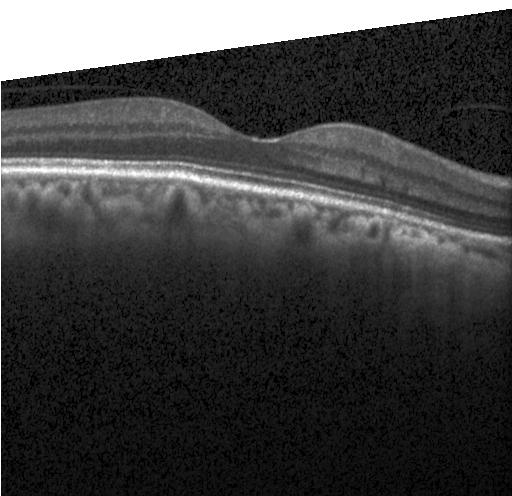
OCT line scan. Acquired on a Heidelberg Spectralis — OCT finding: neither CNV, DME, nor drusen.